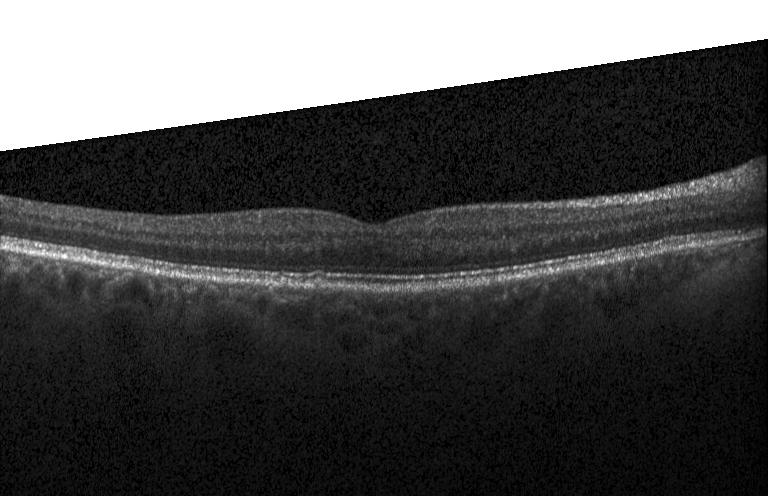

Neither CNV, DME, nor drusen.